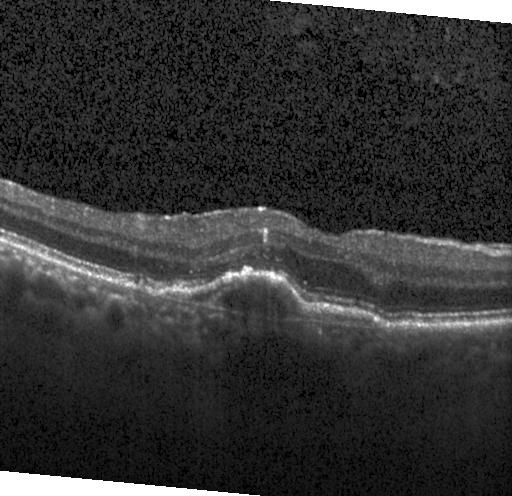

Optical coherence tomography scan; spectral-domain optical coherence tomography
Diagnosis: choroidal neovascularization.